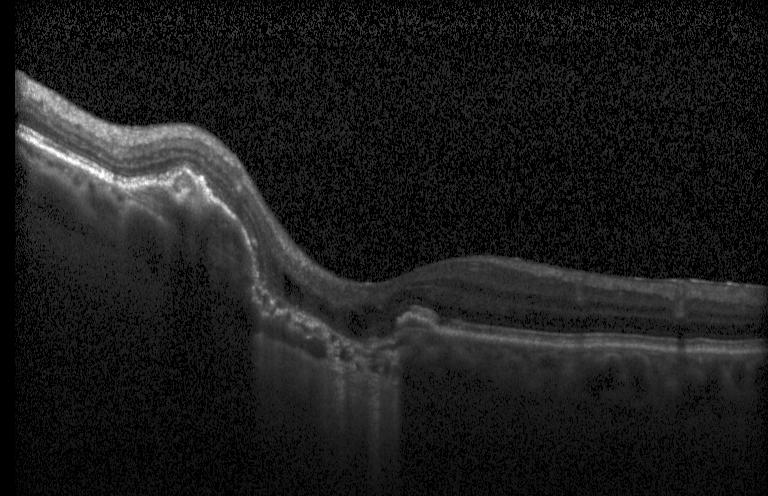 A choroidal neovascular membrane.